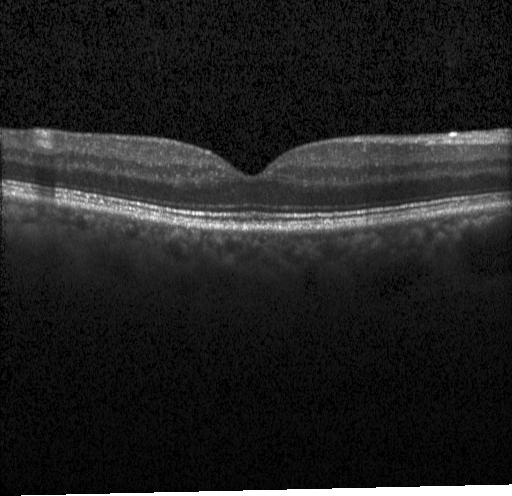

Spectral-domain OCT B-scan: no evidence of CNV, DME, or drusen.